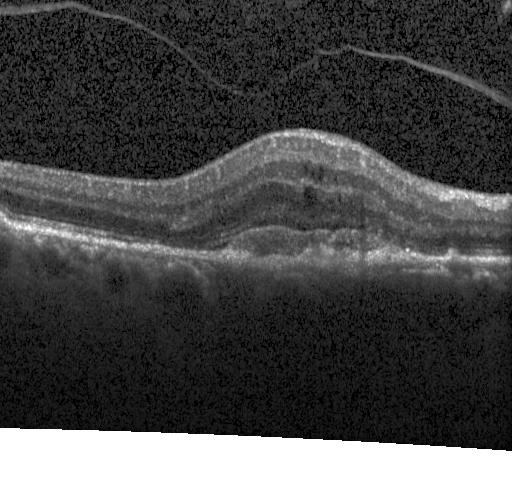
Retinal OCT B-scan. Fovea-centered. Heidelberg Spectralis OCT system. Dx: choroidal neovascularization (CNV).